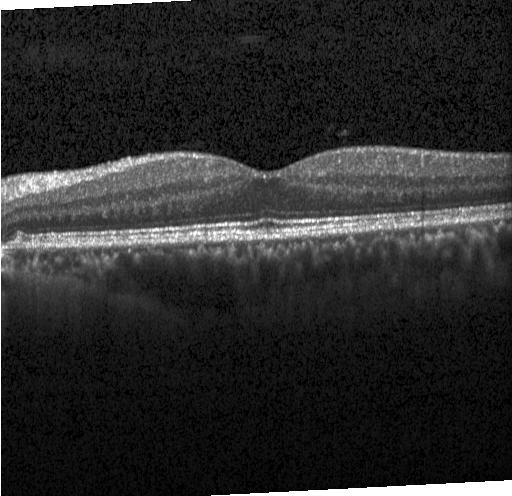
No CNV, DME, or drusen.